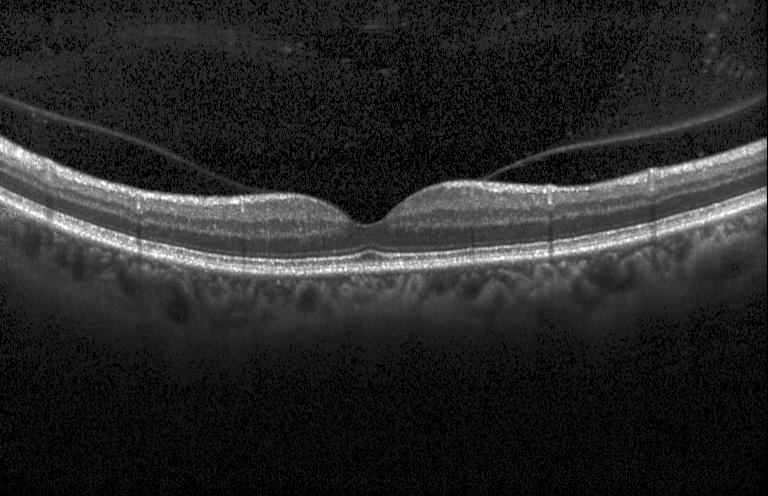 Finding: no CNV, DME, or drusen.